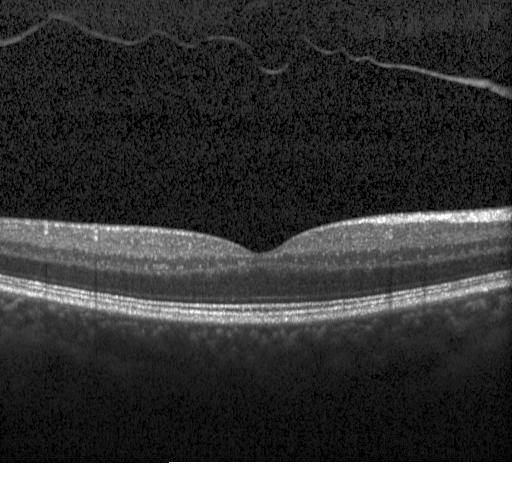 This B-scan demonstrates no choroidal neovascularization, diabetic macular edema, or drusen.